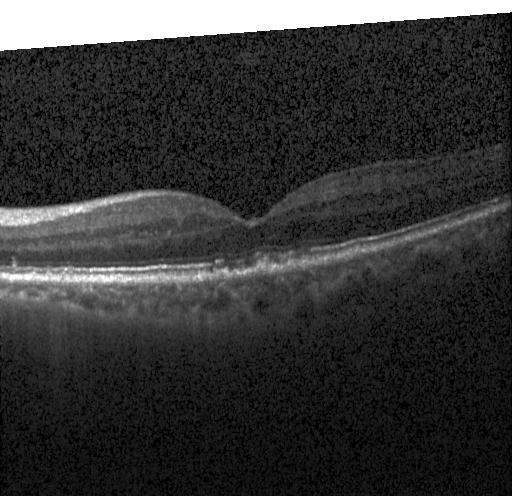
OCT B-scan showing multiple drusen.